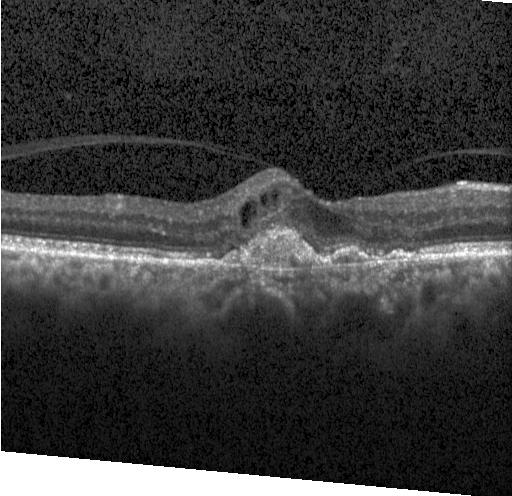 Diagnosis: choroidal neovascularization.